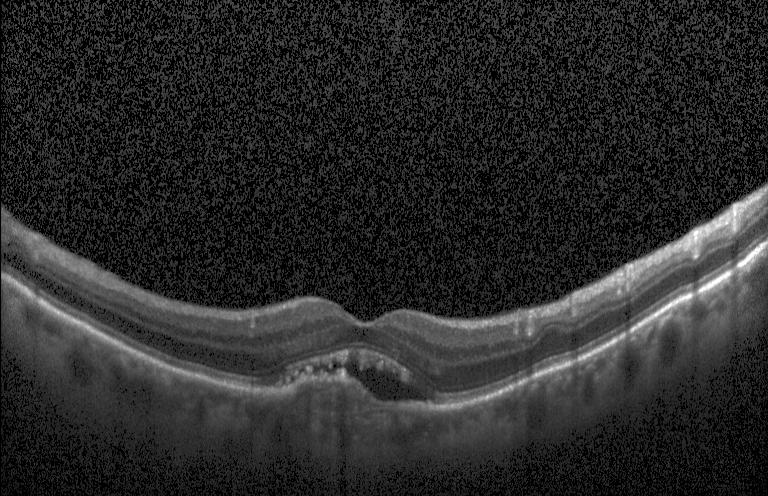

Optical coherence tomography B-scan
Impression: CNV.